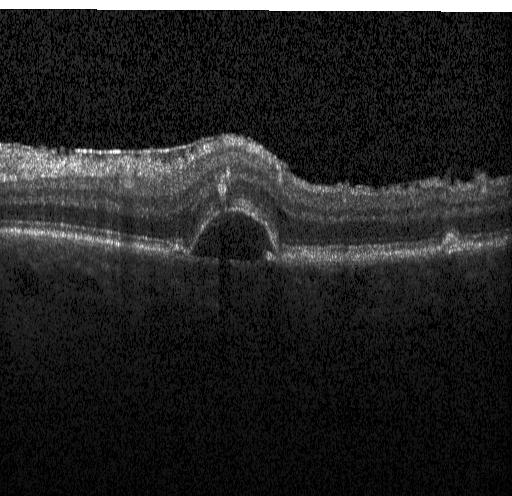 Acquired on a Heidelberg Spectralis; OCT line scan.
Impression: CNV.